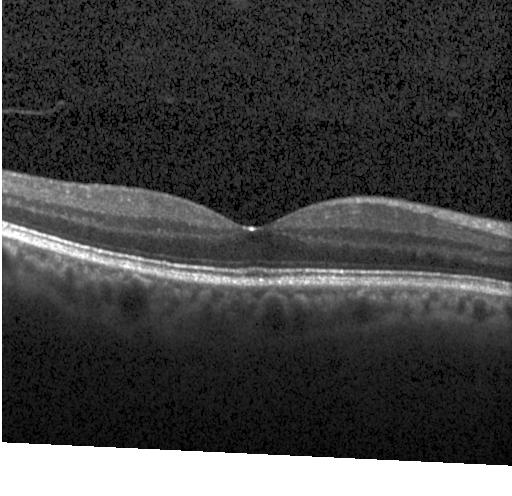 OCT B-scan showing no CNV, DME, or drusen.